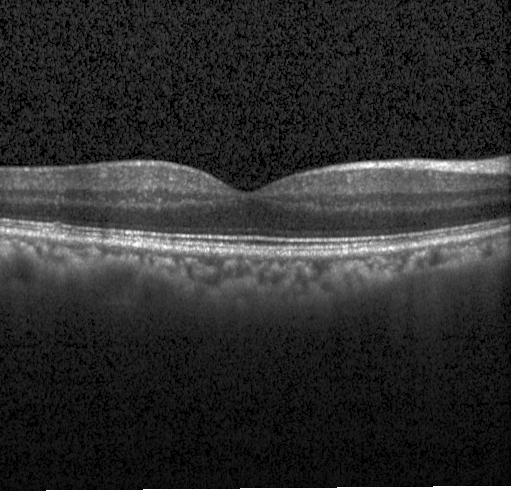

Heidelberg Spectralis OCT system, spectral-domain optical coherence tomography, OCT B-scan. Macular OCT: no evidence of choroidal neovascularization, diabetic macular edema, or drusen.